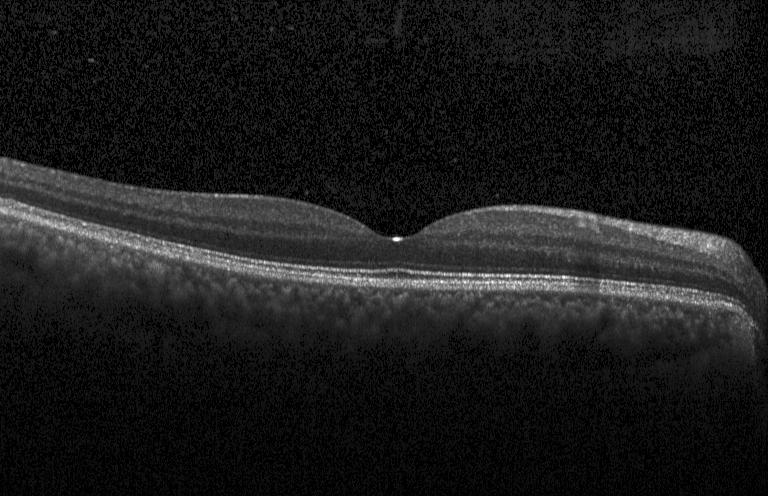 Optical coherence tomography scan · instrument: Heidelberg Spectralis · macular scan · SD-OCT.
Macular OCT: no choroidal neovascularization, diabetic macular edema, or drusen.